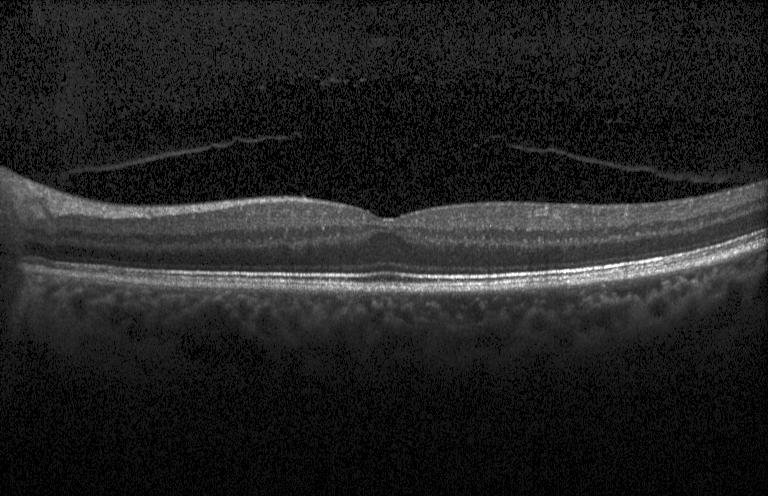 OCT line scan — This B-scan demonstrates no CNV, DME, or drusen.